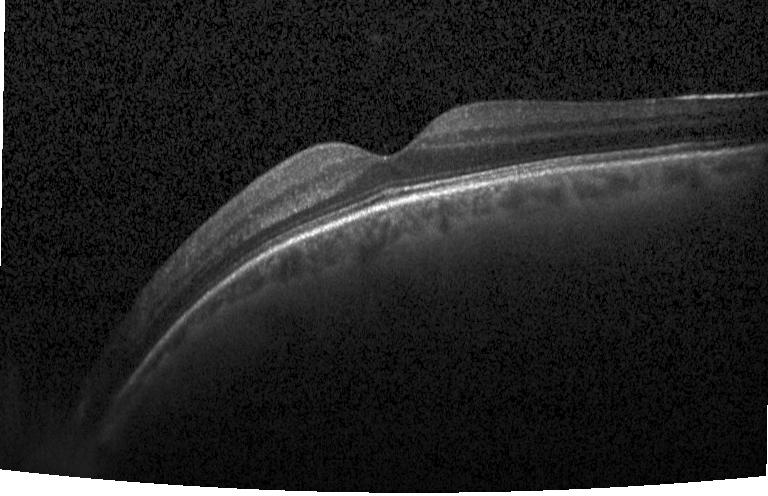 Fovea-centered. Retinal OCT cross-section. Spectral-domain optical coherence tomography — This B-scan demonstrates no choroidal neovascularization, no diabetic macular edema, and no drusen.